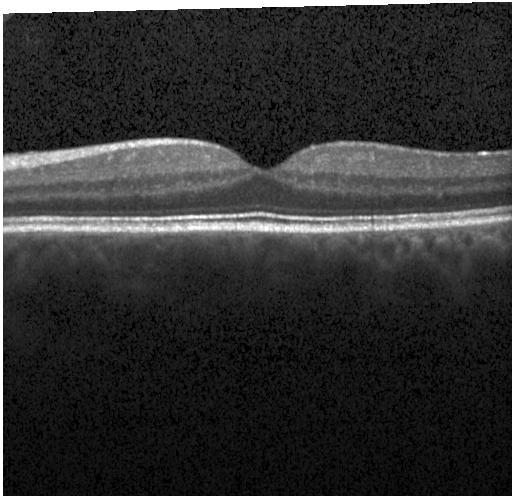
SD-OCT, optical coherence tomography B-scan, instrument: Heidelberg Spectralis.
Diagnosis: neither CNV, DME, nor drusen.